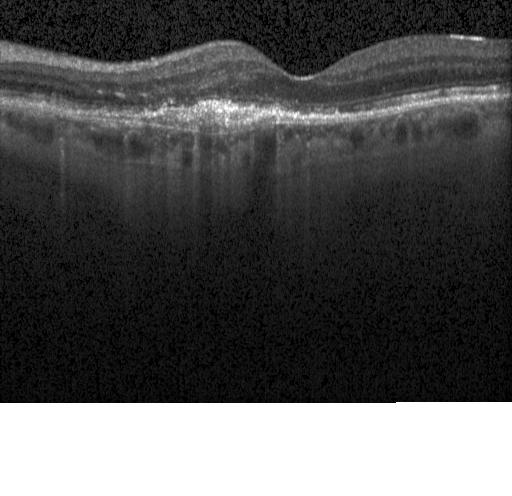

Spectral-domain OCT. OCT B-scan
Diagnosis: choroidal neovascularization (CNV).